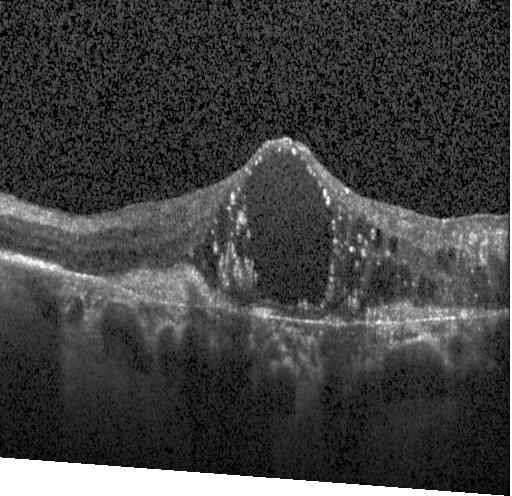 Diagnosis: a choroidal neovascular membrane.